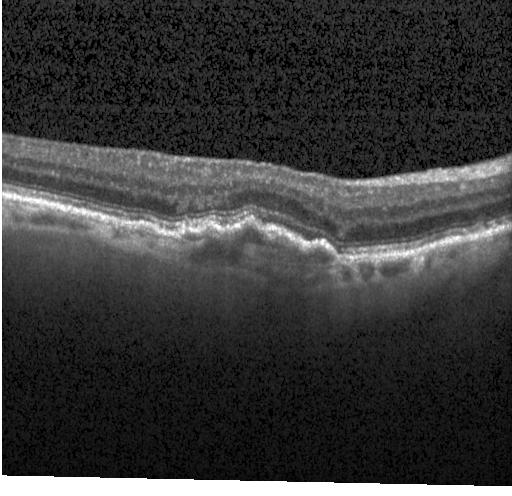 Instrument: Heidelberg Spectralis; SD-OCT; OCT line scan
Assessment: CNV.